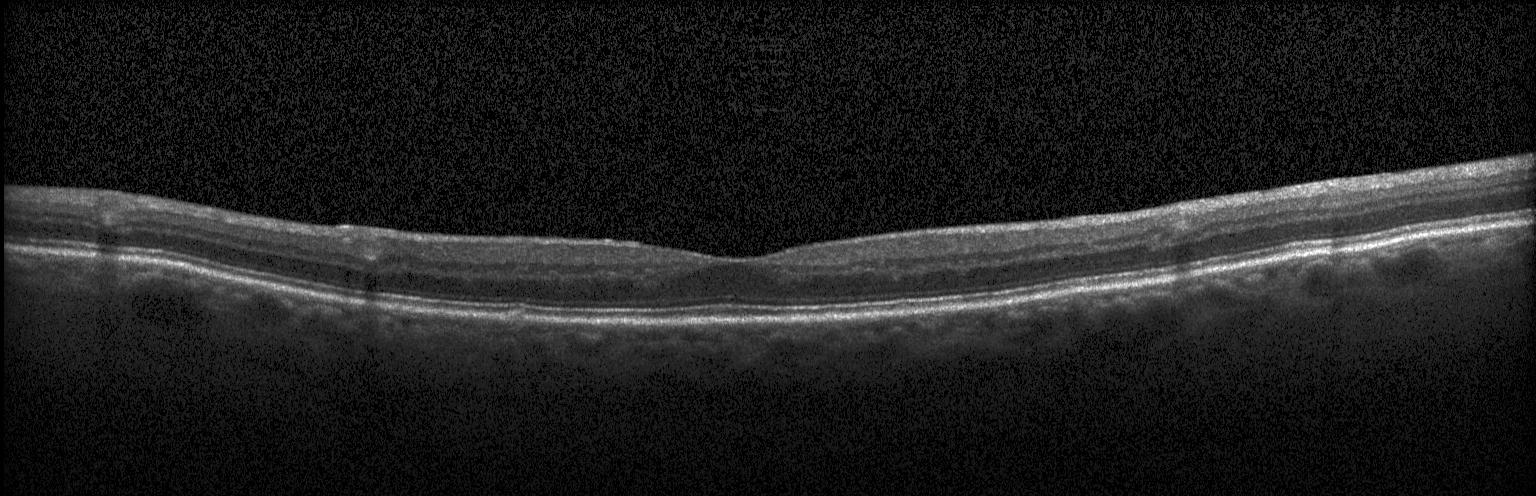
Through the macula; OCT B-scan. Impression: neither CNV, DME, nor drusen.